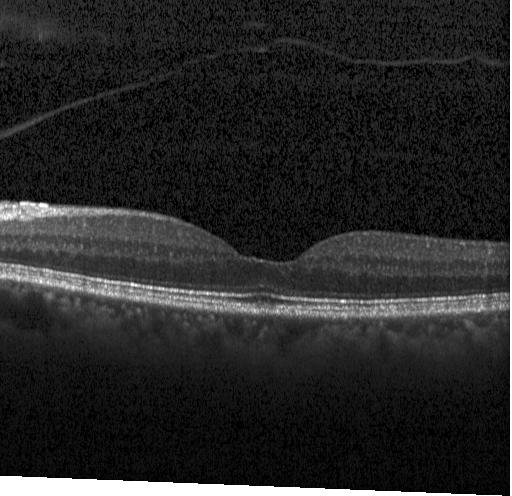
Retinal OCT cross-section
Macular OCT: no choroidal neovascularization, diabetic macular edema, or drusen.